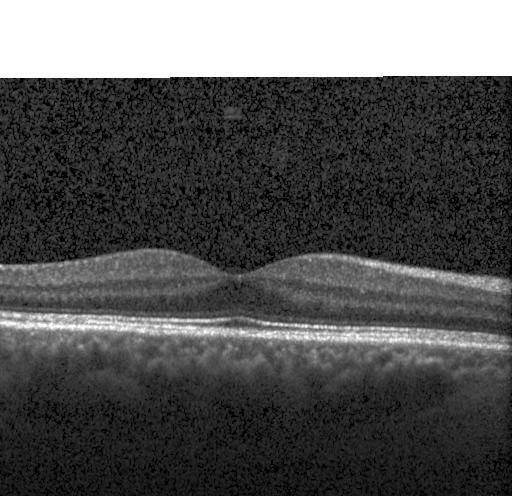 No CNV, no DME, and no drusen.